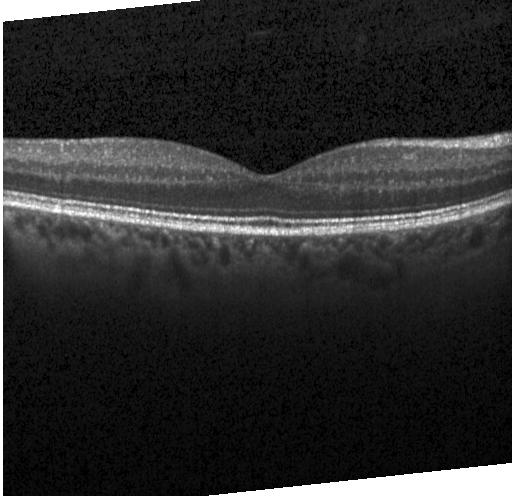 Heidelberg Spectralis; spectral-domain optical coherence tomography; optical coherence tomography B-scan; through the macula — Diagnosis: no evidence of CNV, DME, or drusen.